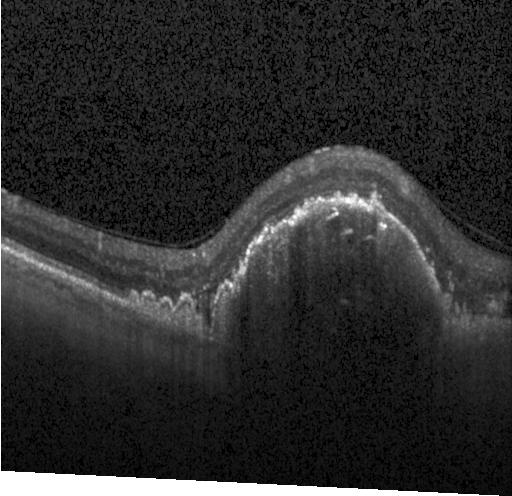

Macular OCT: a choroidal neovascular membrane.